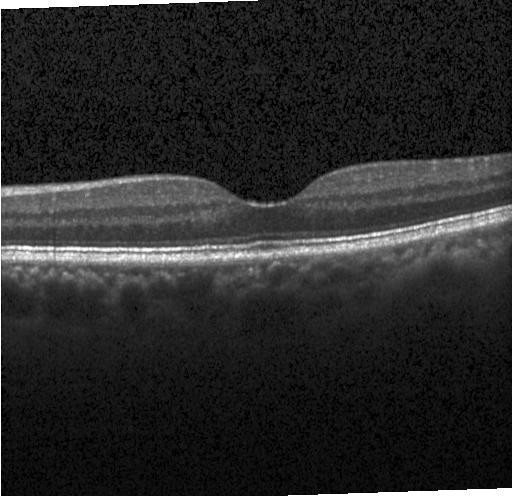
Retinal OCT B-scan, spectral-domain OCT.
Diagnosis: neither choroidal neovascularization, diabetic macular edema, nor drusen.